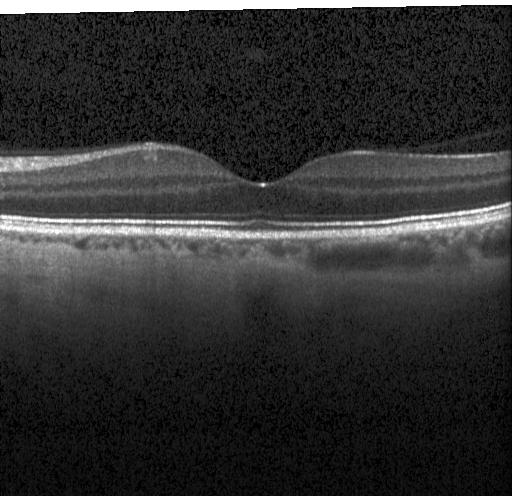
Heidelberg Spectralis; macular scan; OCT B-scan; SD-OCT
Diagnosis: no choroidal neovascularization, diabetic macular edema, or drusen.